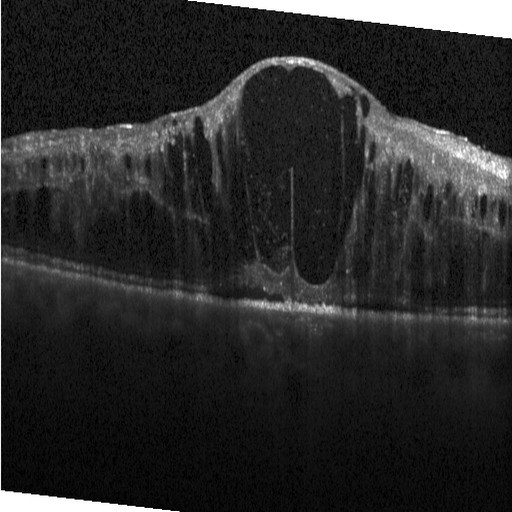

Optical coherence tomography B-scan.
Macular OCT: diabetic macular edema.